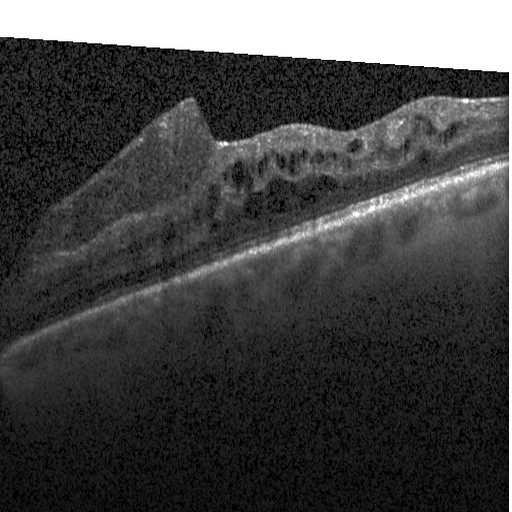
Instrument: Heidelberg Spectralis · retinal OCT cross-section · centered on the fovea.
Impression: diabetic macular edema.